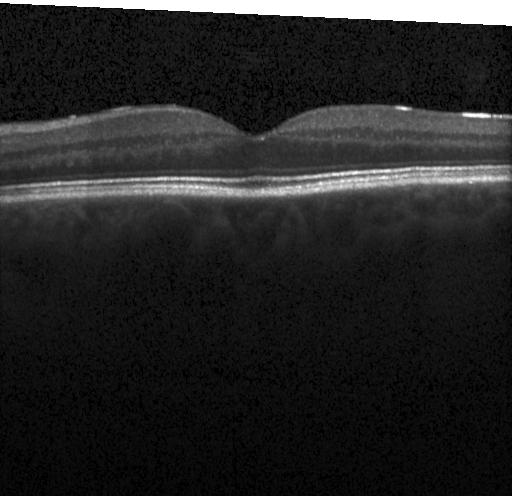

OCT finding: no choroidal neovascularization, no diabetic macular edema, and no drusen.